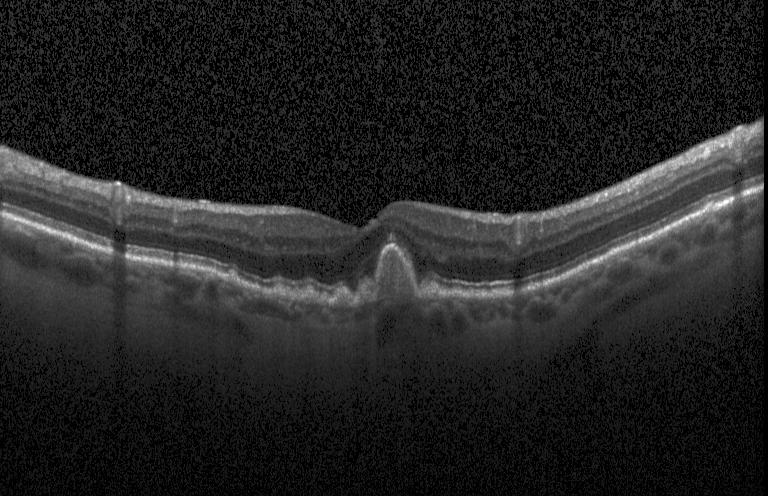

Optical coherence tomography B-scan
Assessment: drusen.